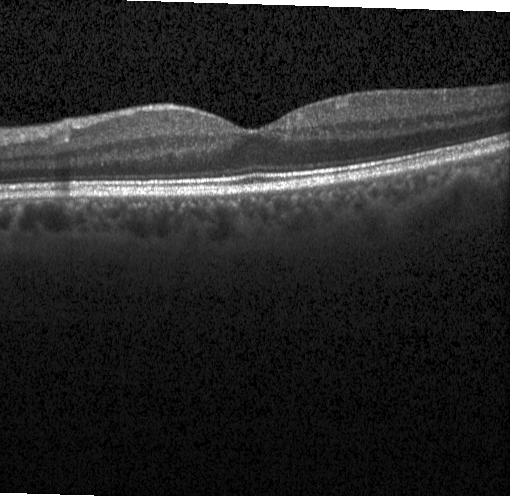 Finding: no choroidal neovascularization, diabetic macular edema, or drusen.